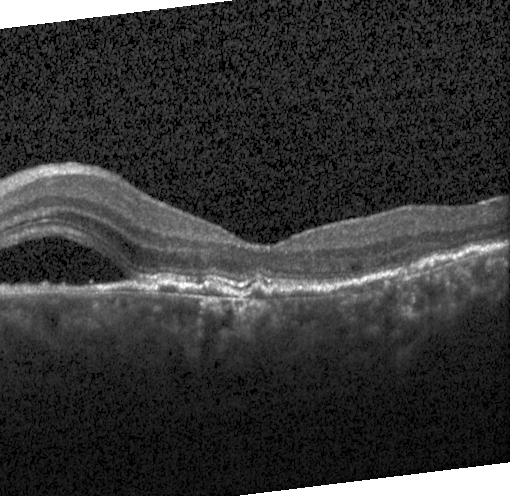
Spectral-domain OCT, OCT line scan, centered on the fovea, acquired on a Heidelberg Spectralis
Impression: a choroidal neovascular membrane.